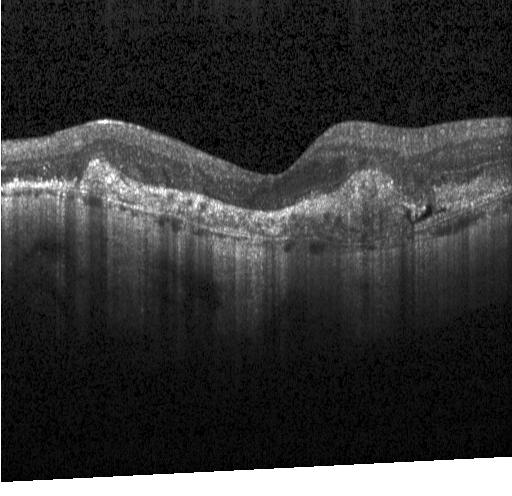 OCT B-scan. Heidelberg Spectralis
Assessment: CNV.